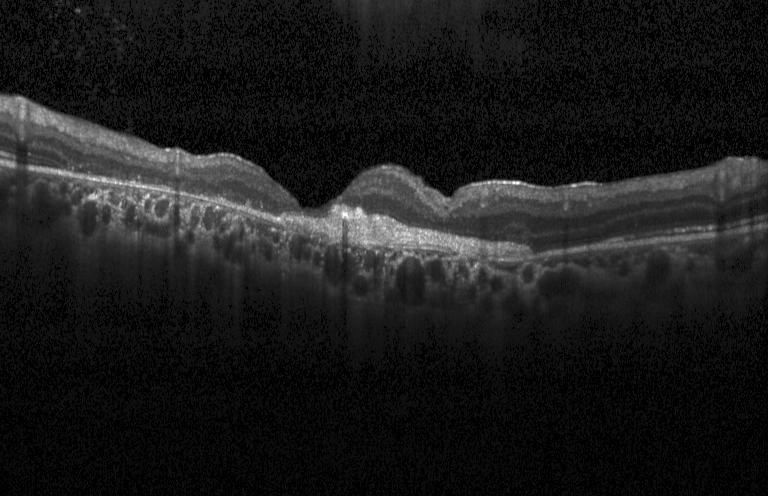

OCT B-scan showing a choroidal neovascular membrane.